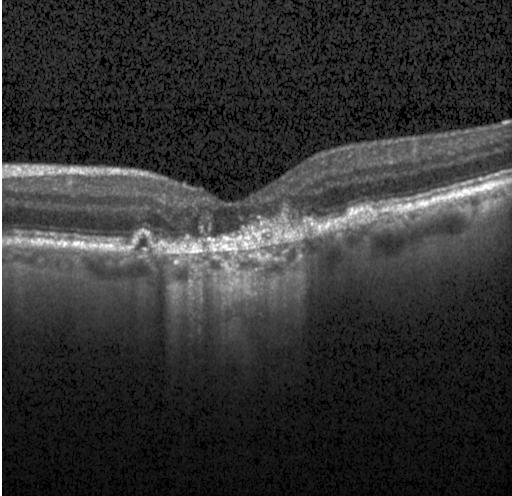
OCT finding: a choroidal neovascular membrane.